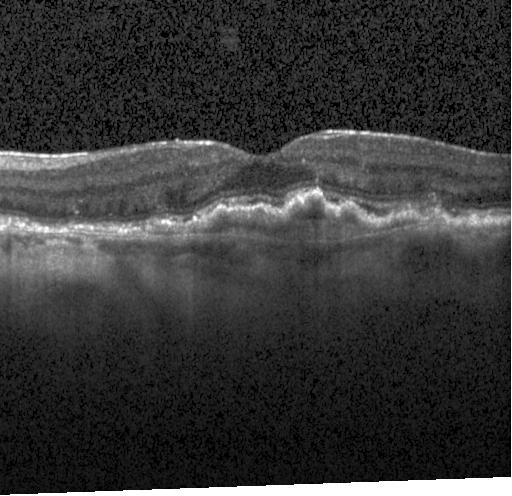
Retinal OCT B-scan · acquired on a Heidelberg Spectralis · through the macula.
Finding: a choroidal neovascular membrane.